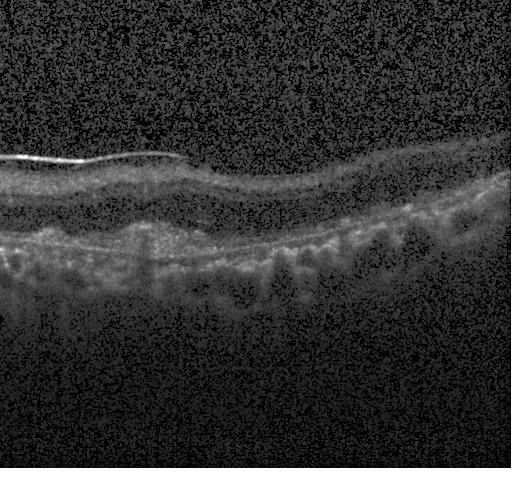

Instrument: Heidelberg Spectralis, optical coherence tomography scan, SD-OCT
Impression: choroidal neovascularization (CNV).